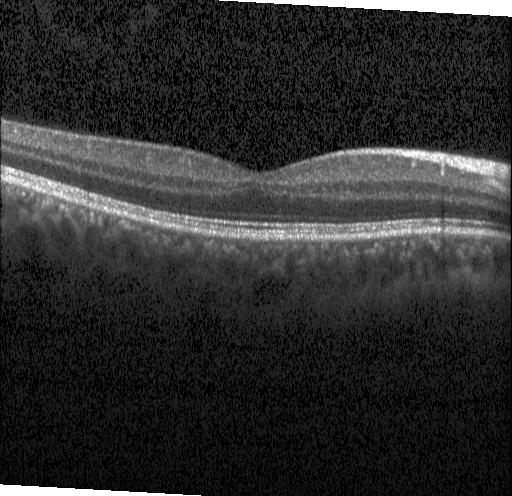 SD-OCT; through the macula; OCT B-scan. Impression: no evidence of choroidal neovascularization, diabetic macular edema, or drusen.